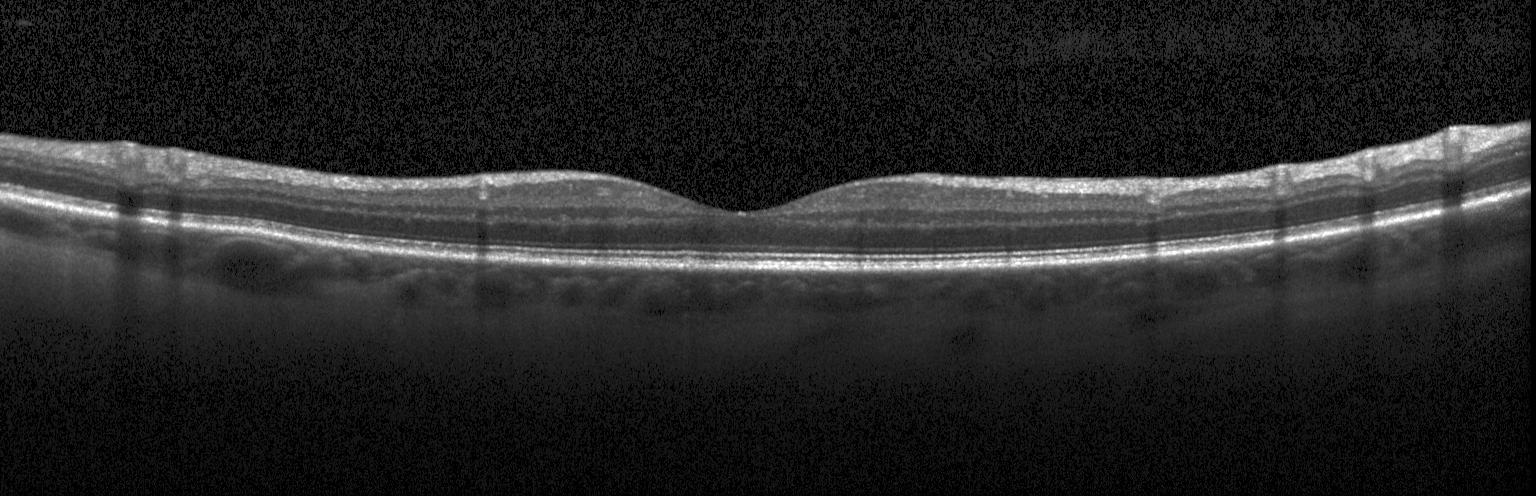 OCT B-scan; spectral-domain optical coherence tomography; acquired on a Heidelberg Spectralis; macular scan
Finding: no choroidal neovascularization, diabetic macular edema, or drusen.